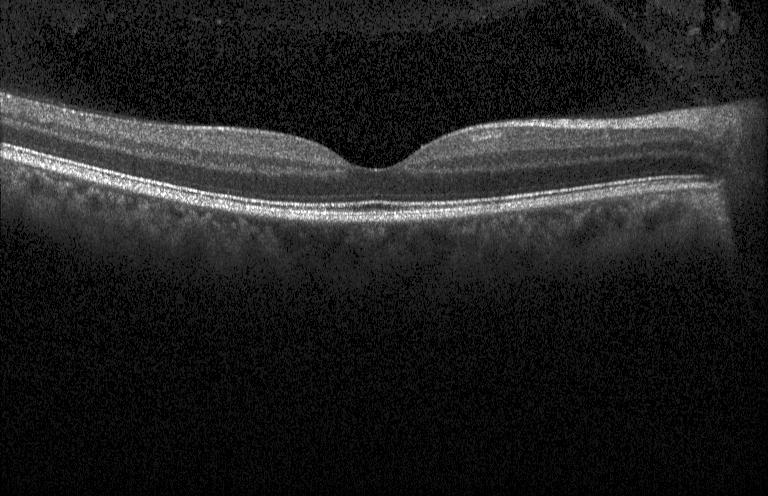 OCT B-scan; SD-OCT; through the macula; acquired on a Heidelberg Spectralis.
Dx: no evidence of CNV, DME, or drusen.